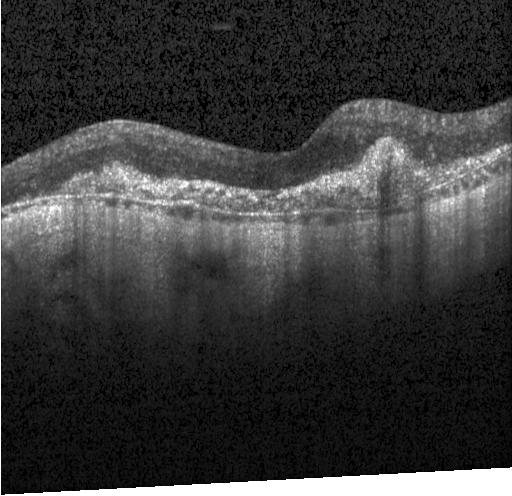 OCT B-scan showing CNV.